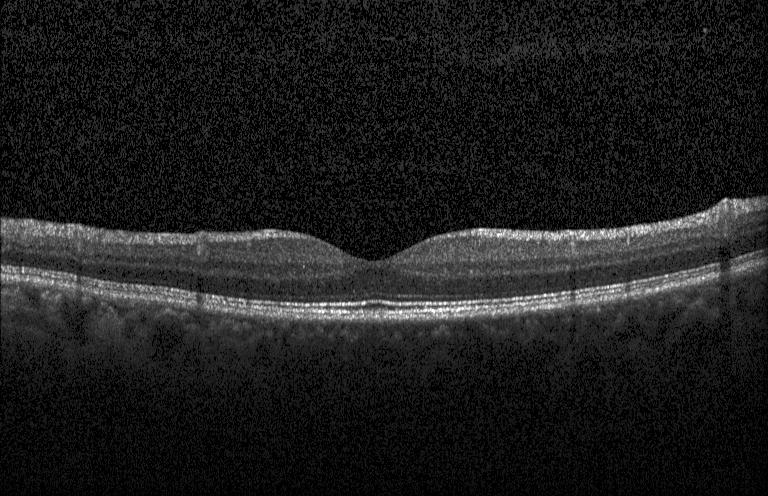

Optical coherence tomography scan.
Macular OCT: neither CNV, DME, nor drusen.